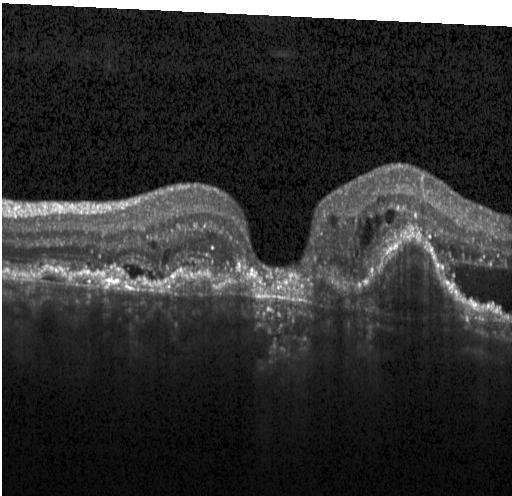

SD-OCT. Macular scan. Heidelberg Spectralis OCT system. Optical coherence tomography B-scan.
Macular OCT: CNV.